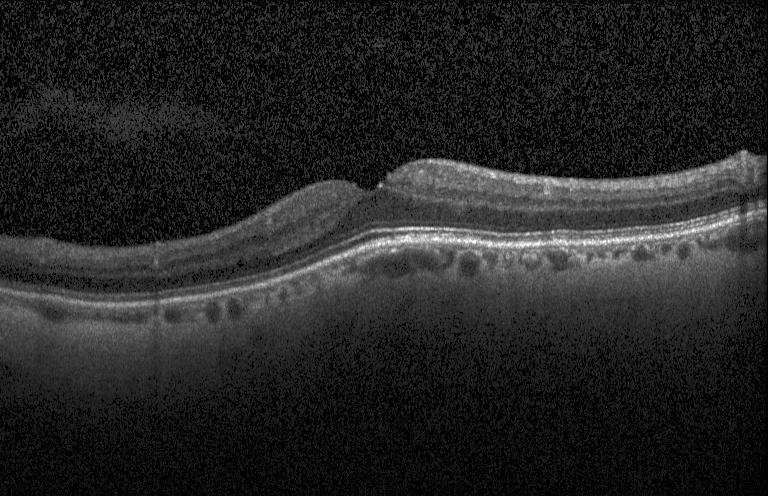

Spectral-domain optical coherence tomography, optical coherence tomography B-scan, horizontal scan through the fovea
The scan shows no CNV, DME, or drusen.